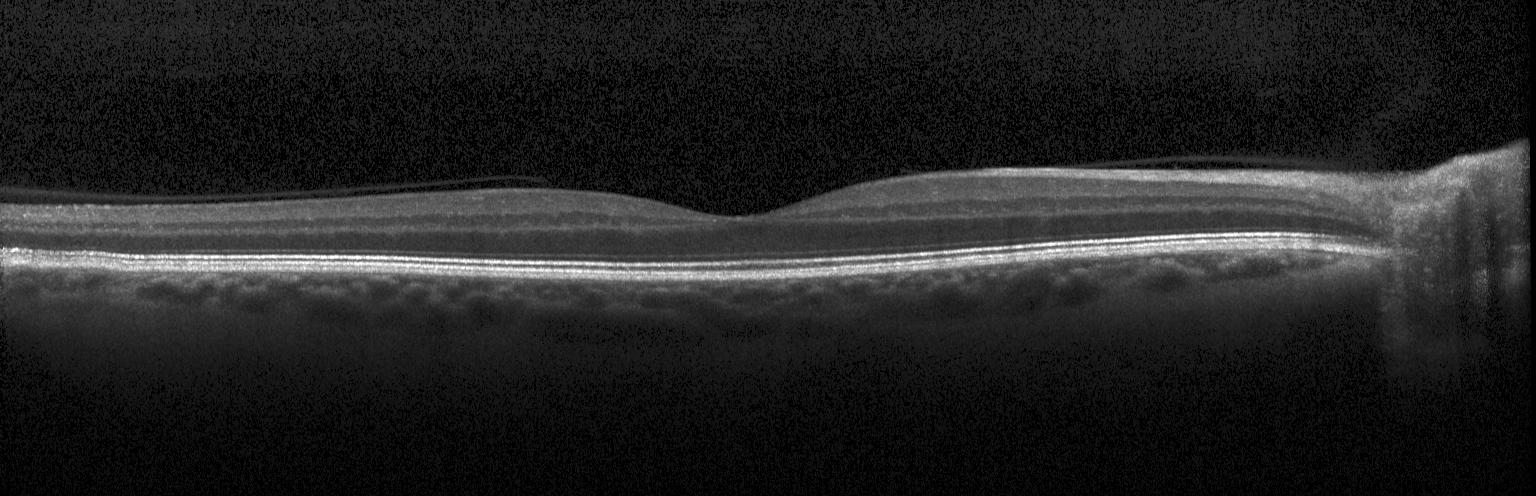 Retinal OCT B-scan. Diagnosis: no evidence of choroidal neovascularization, diabetic macular edema, or drusen.